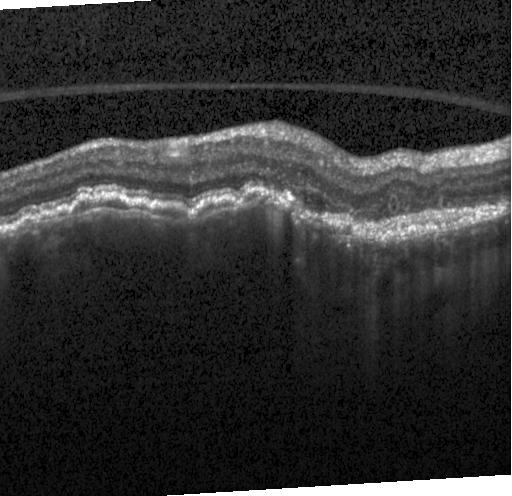

Spectral-domain optical coherence tomography · Heidelberg Spectralis · horizontal scan through the fovea · retinal OCT cross-section. Finding: a choroidal neovascular membrane.